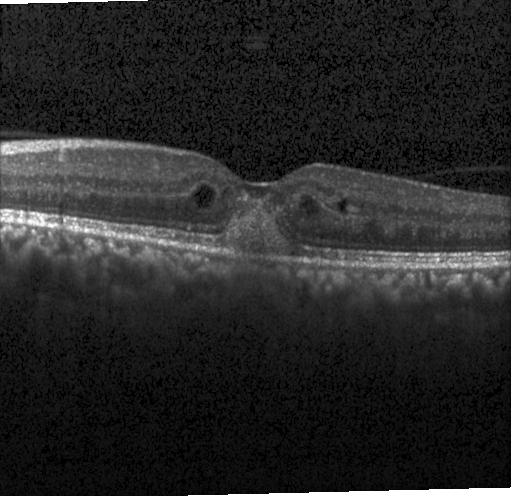 Instrument: Heidelberg Spectralis. OCT line scan.
Impression: choroidal neovascularization (CNV).